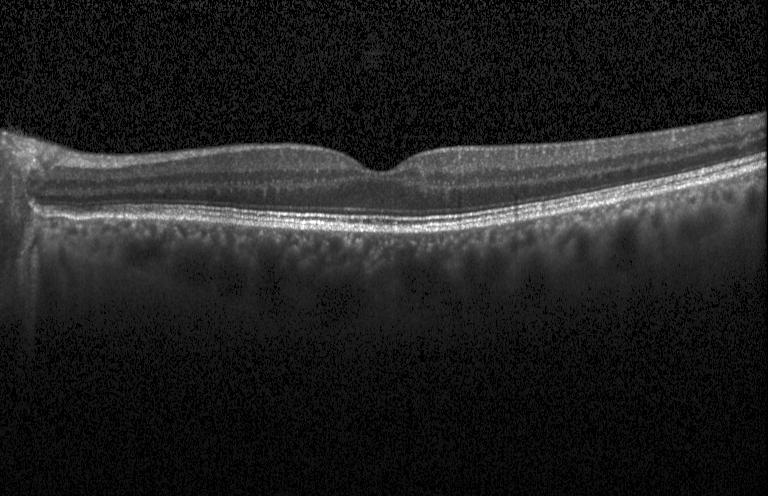 Optical coherence tomography B-scan — Impression: neither choroidal neovascularization, diabetic macular edema, nor drusen.